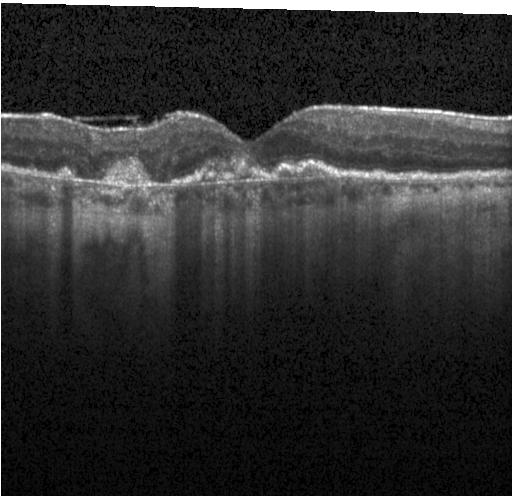 OCT B-scan showing choroidal neovascularization (CNV).